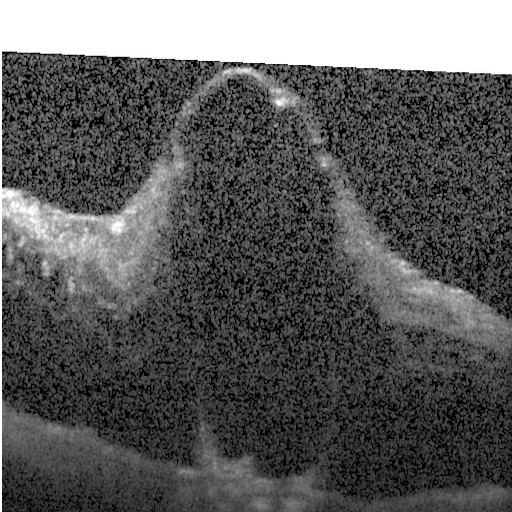

Optical coherence tomography B-scan · macular scan · SD-OCT · acquired on a Heidelberg Spectralis. Assessment: diabetic macular edema (DME).